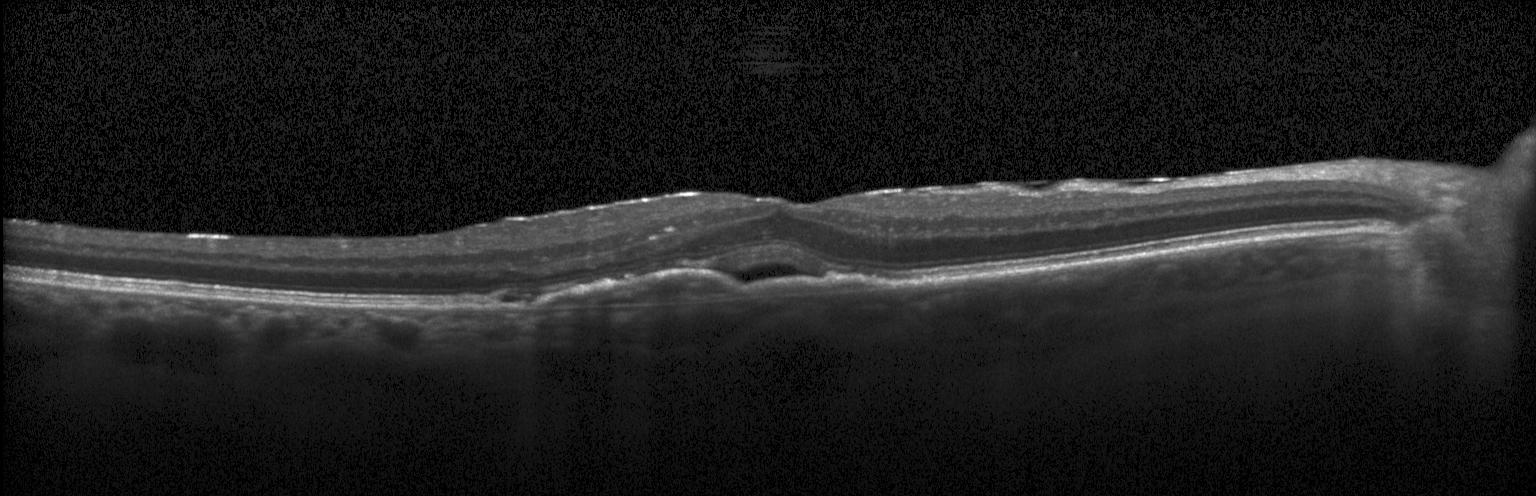
Centered on the fovea. Optical coherence tomography B-scan. Instrument: Heidelberg Spectralis.
Impression: CNV.